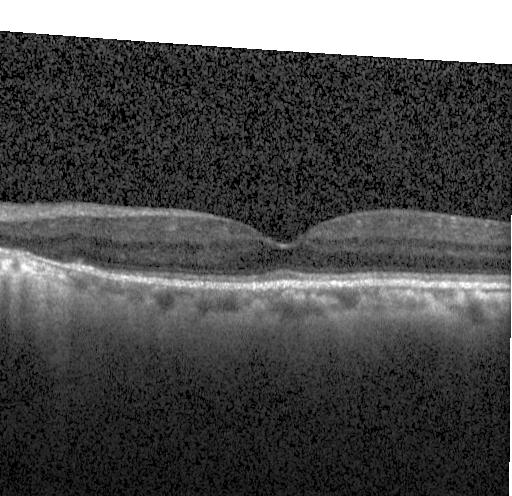 Heidelberg Spectralis OCT system, spectral-domain optical coherence tomography, horizontal scan through the fovea, OCT B-scan — This B-scan demonstrates no evidence of choroidal neovascularization, diabetic macular edema, or drusen.